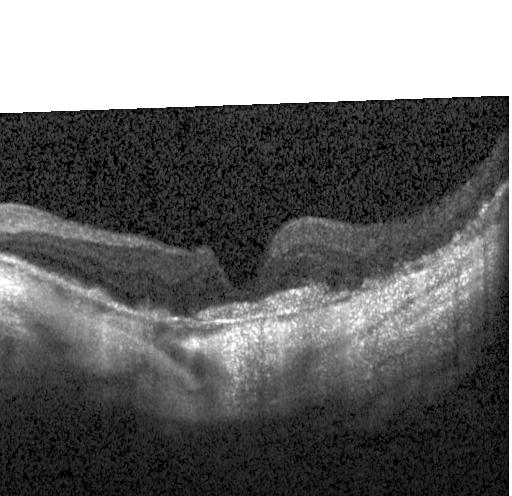

Retinal OCT cross-section showing a choroidal neovascular membrane.